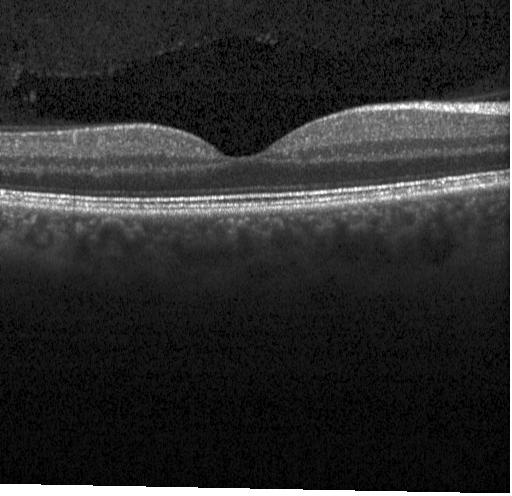 Through the macula, optical coherence tomography scan, acquired on a Heidelberg Spectralis — This B-scan demonstrates no choroidal neovascularization, diabetic macular edema, or drusen.